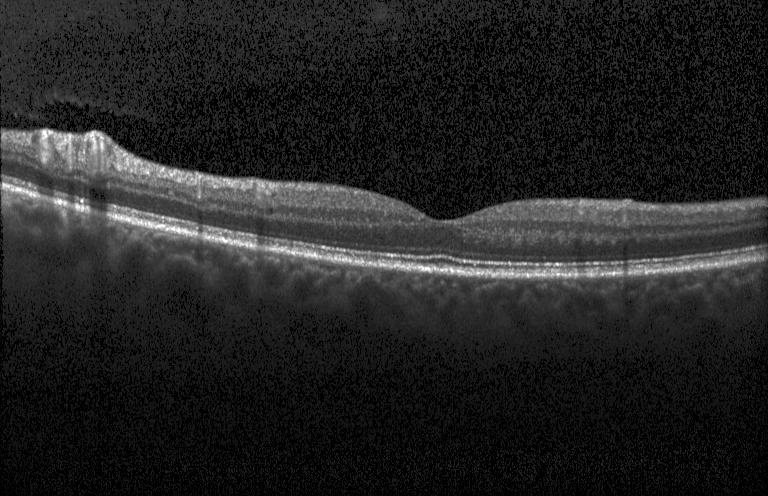

OCT finding: no CNV, no DME, and no drusen.